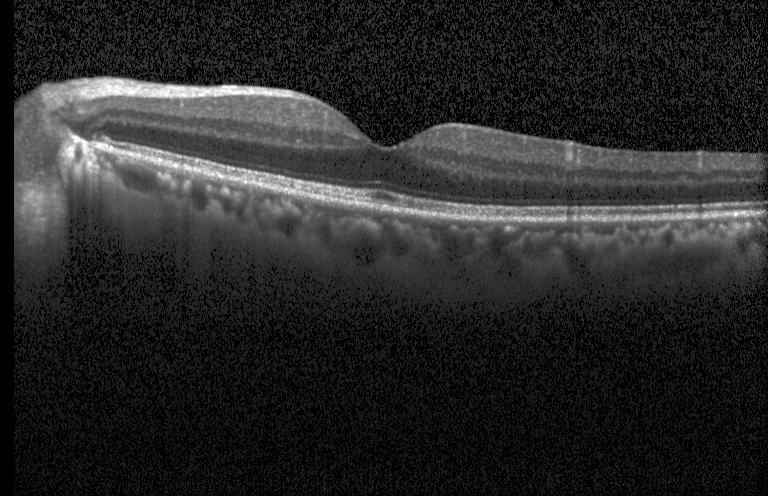

Diagnosis: no choroidal neovascularization, diabetic macular edema, or drusen.